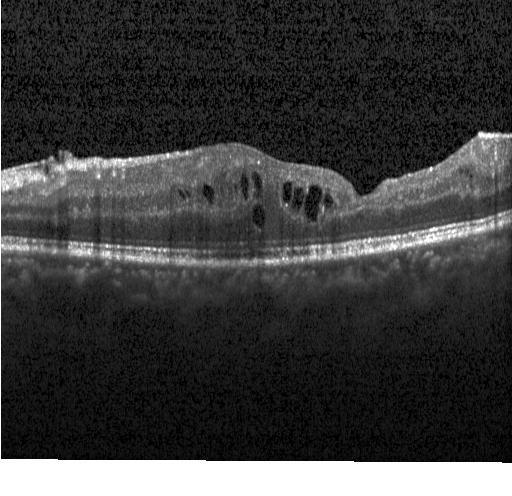

Spectral-domain OCT. Horizontal scan through the fovea. Optical coherence tomography B-scan.
Impression: diabetic macular edema (DME).